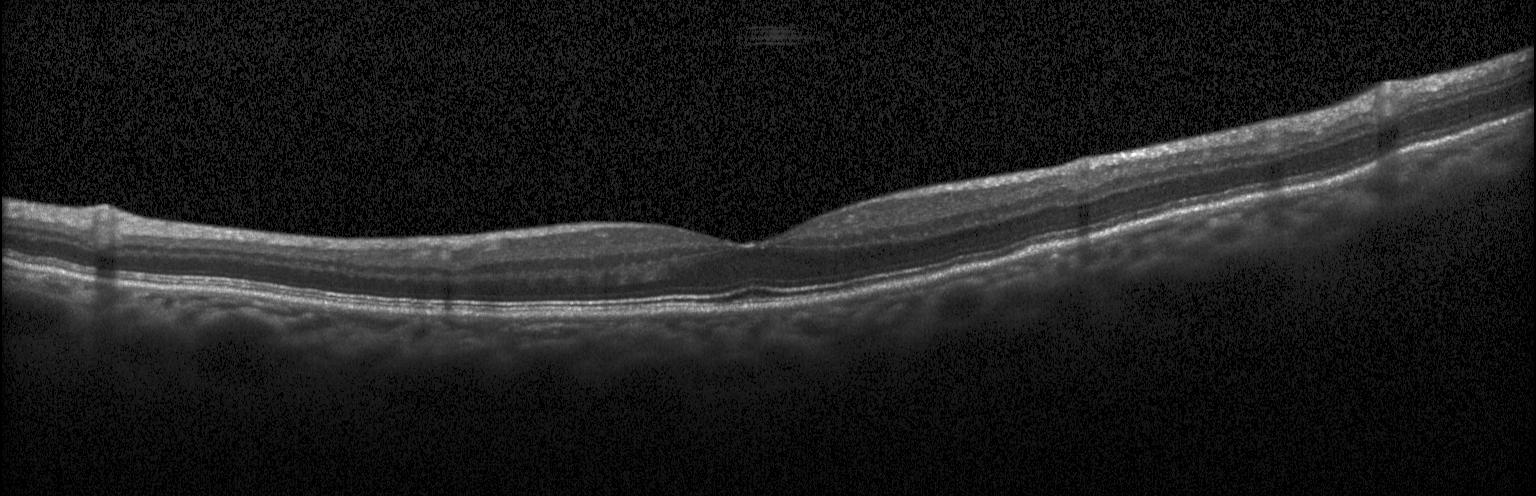 Retinal OCT cross-section
Impression: neither CNV, DME, nor drusen.